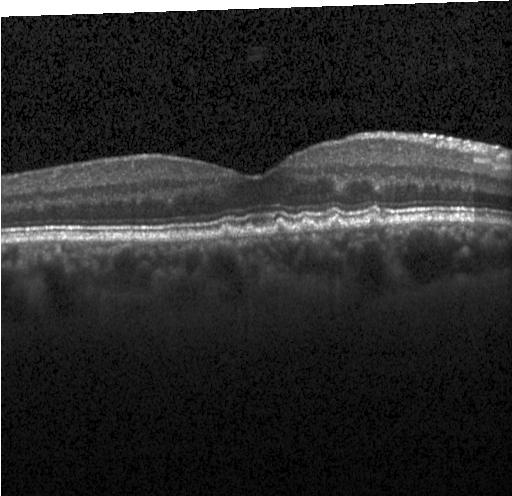 Optical coherence tomography scan. Impression: drusen.